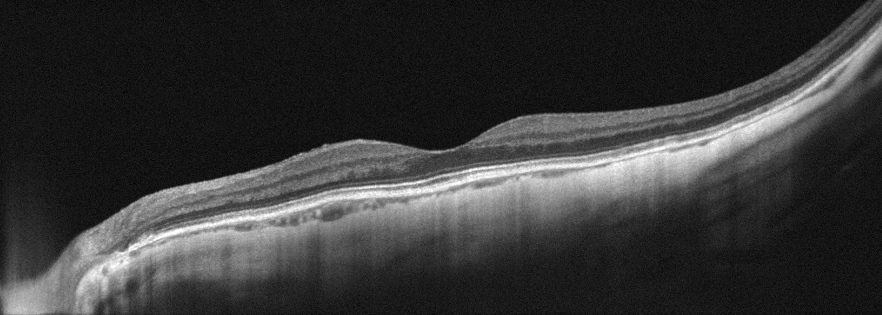

OS, OCT B-scan, instrument: Optovue Avanti RTVue XR — Finding: no AMD, DME, ERM, RAO, RVO, or VID.